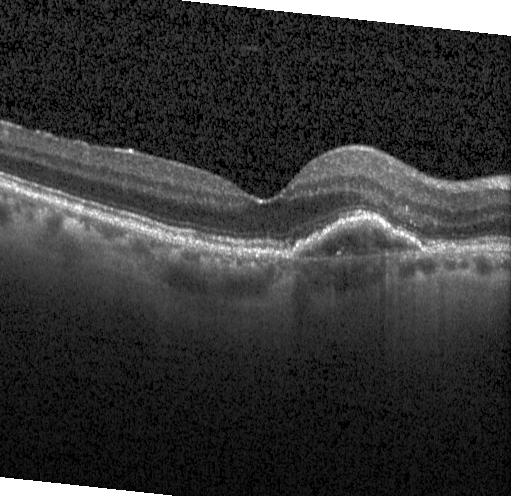 Impression: CNV.